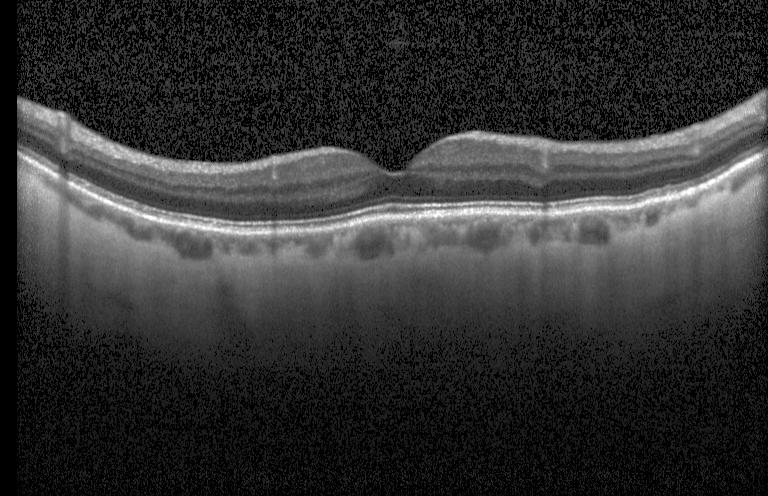

OCT finding: no CNV, DME, or drusen.